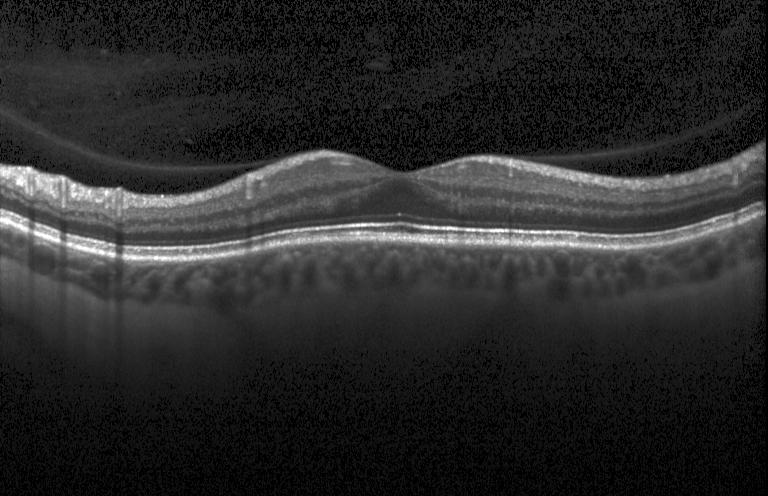
Optical coherence tomography B-scan; centered on the fovea. Macular OCT: no choroidal neovascularization, diabetic macular edema, or drusen.